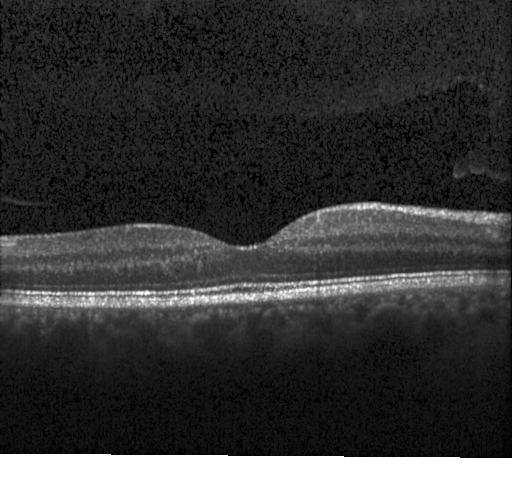

Optical coherence tomography scan. Instrument: Heidelberg Spectralis — Finding: no evidence of CNV, DME, or drusen.